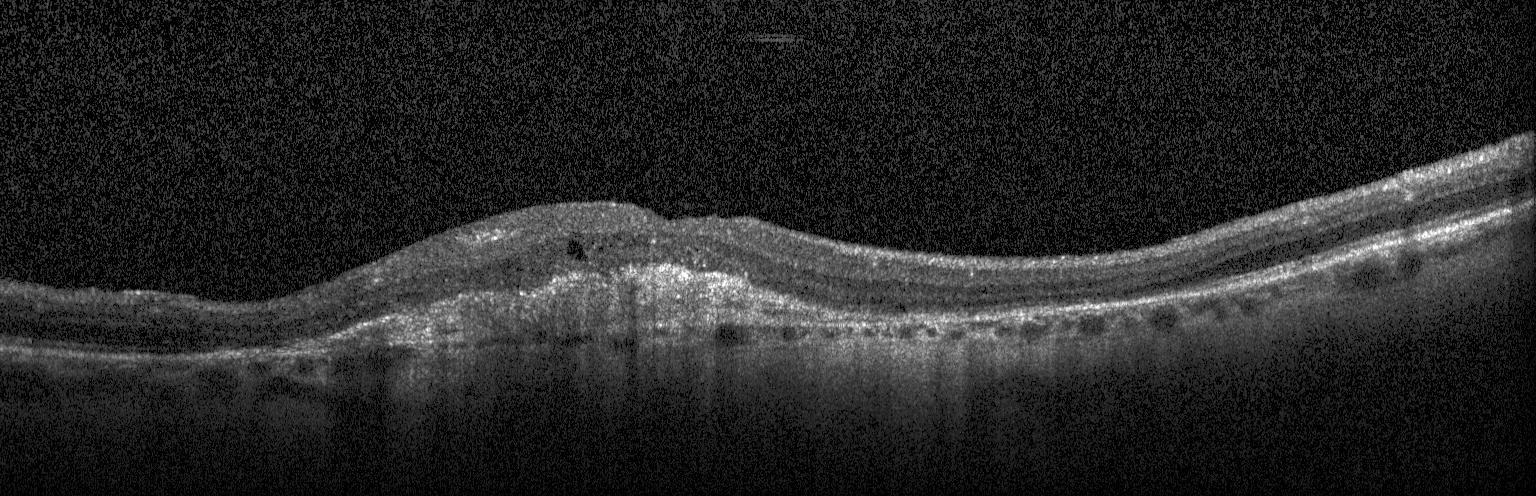
Through the macula, Heidelberg Spectralis, retinal OCT B-scan.
Finding: a choroidal neovascular membrane.